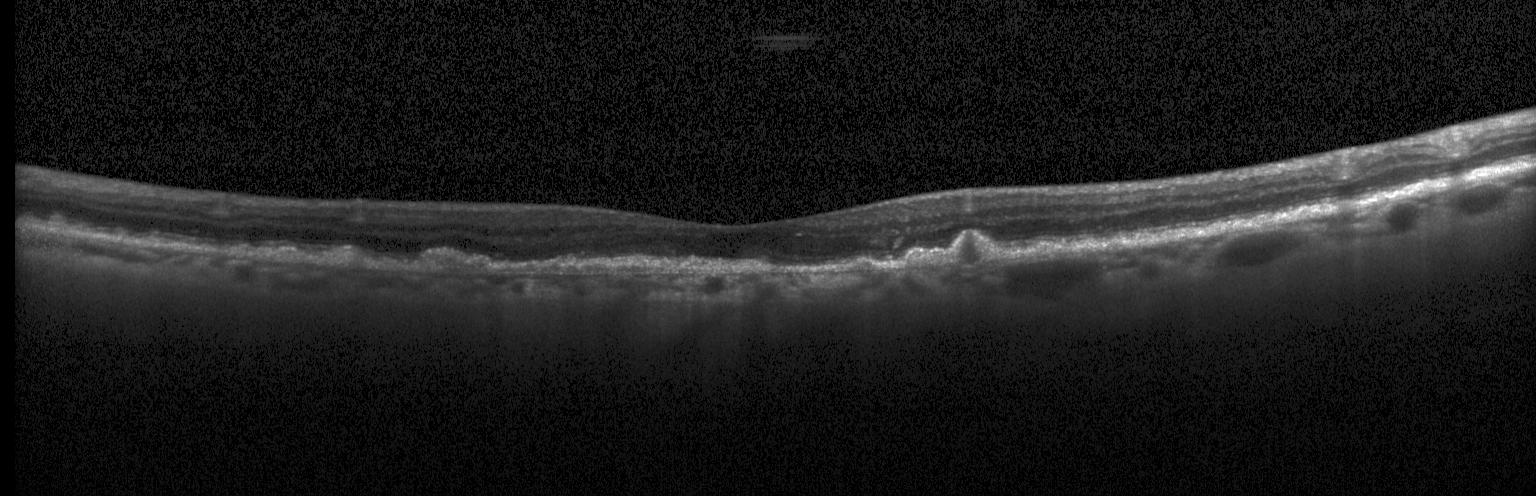

Retinal OCT cross-section
Choroidal neovascularization.